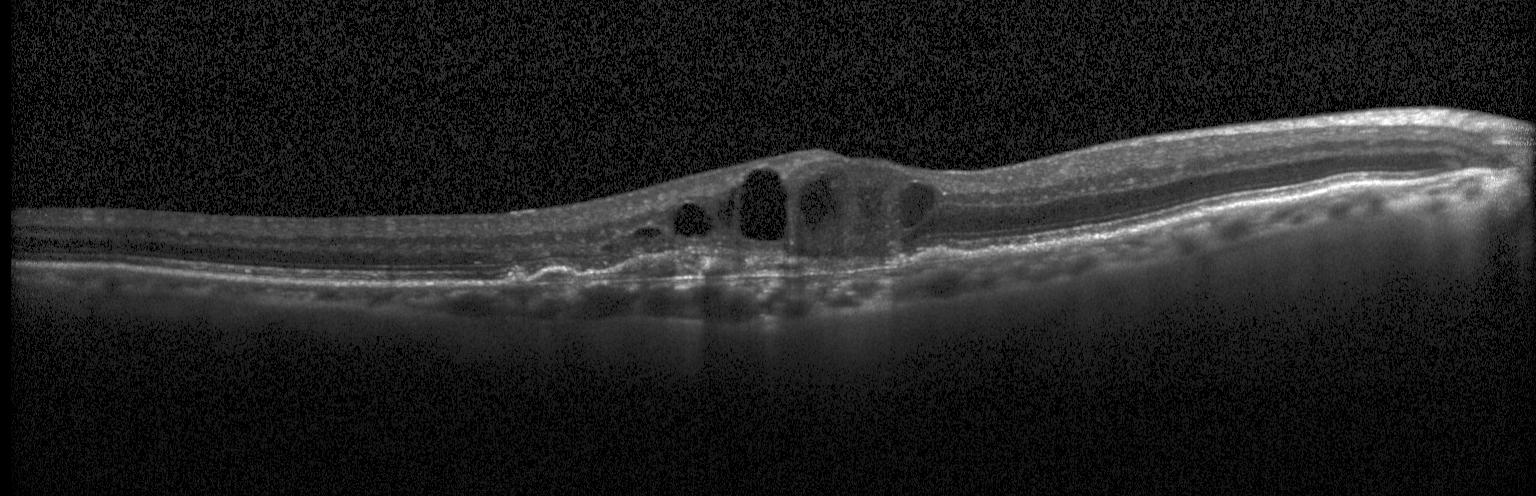 Impression: choroidal neovascularization.